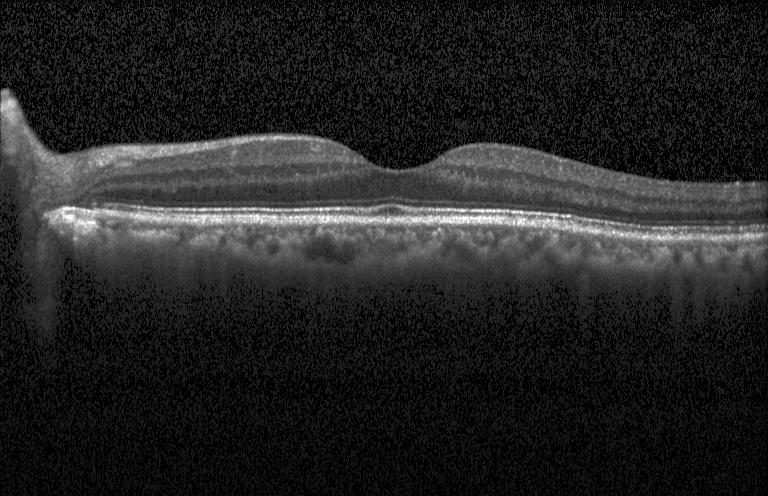 Diagnosis: no evidence of choroidal neovascularization, diabetic macular edema, or drusen.